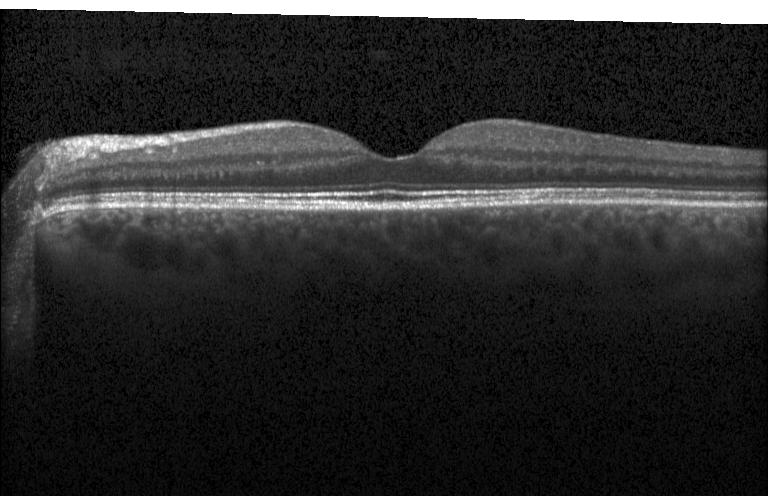

Assessment: no CNV, DME, or drusen.